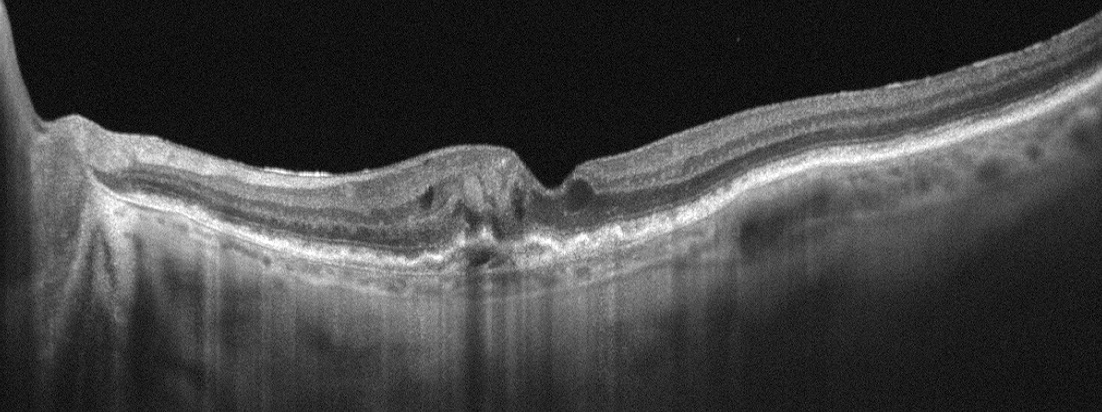 Optical coherence tomography B-scan. OCT finding: AMD.